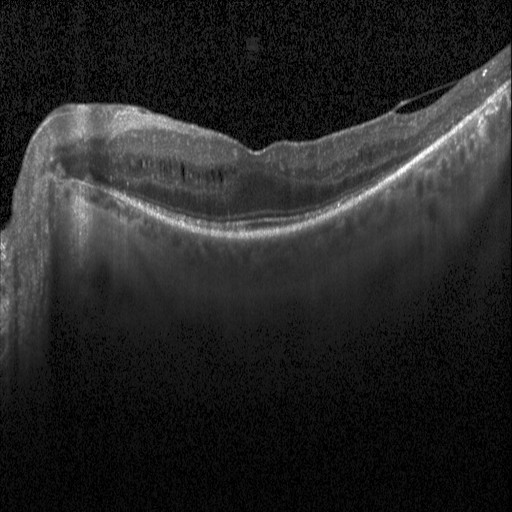 OCT line scan, SD-OCT, through the macula, Heidelberg Spectralis OCT system — Diagnosis: DME.